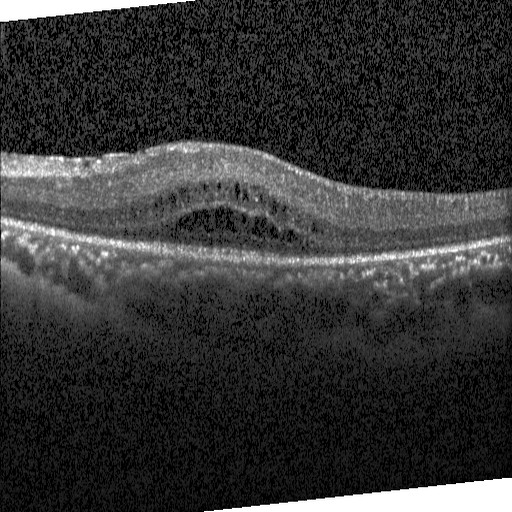
Diagnosis: diabetic macular edema.